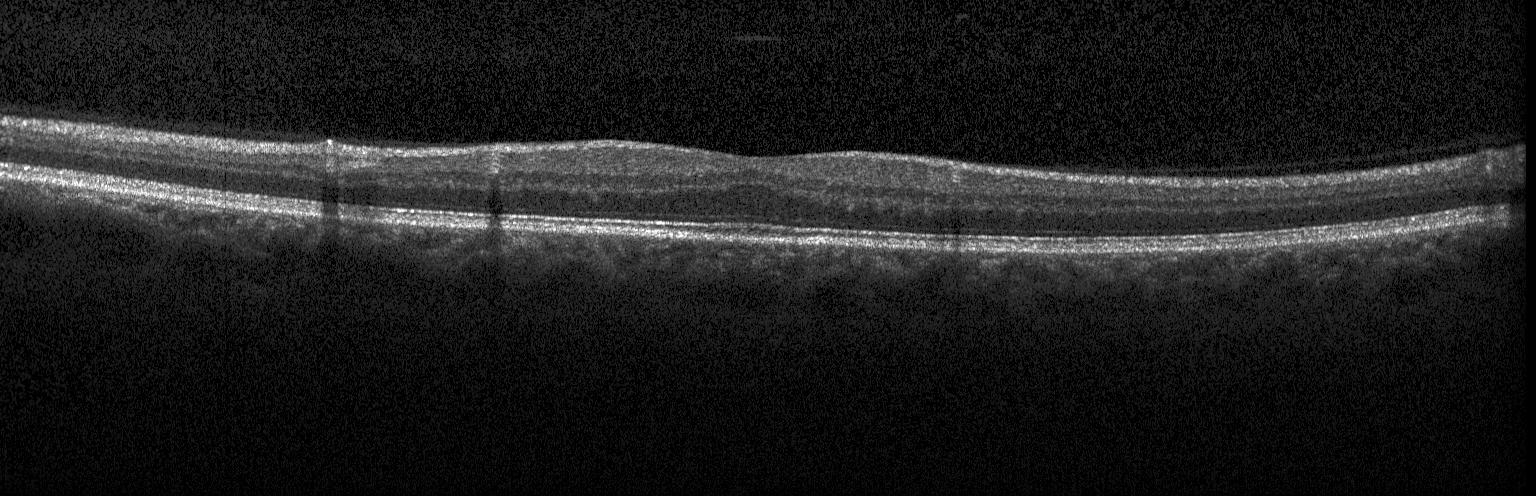 Impression: no choroidal neovascularization, diabetic macular edema, or drusen.